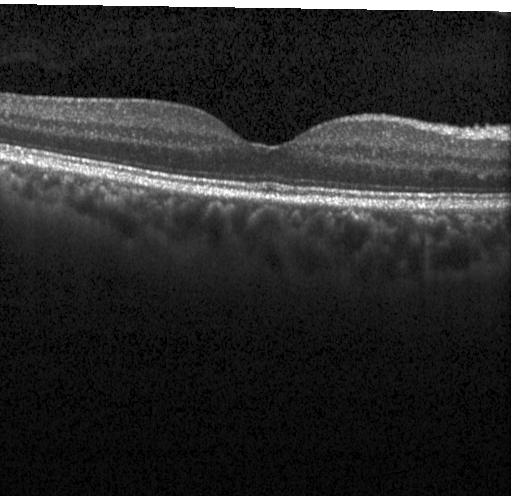 Horizontal scan through the fovea; spectral-domain OCT; OCT B-scan — Assessment: neither CNV, DME, nor drusen.